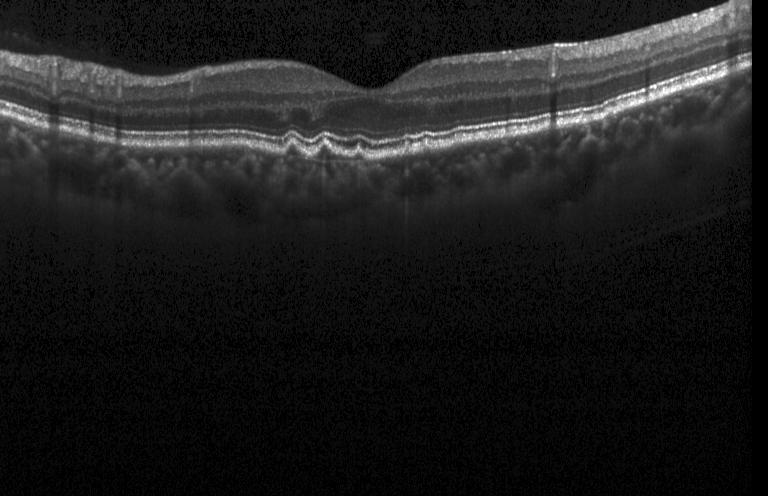

Optical coherence tomography scan, spectral-domain optical coherence tomography, instrument: Heidelberg Spectralis, macular scan
Diagnosis: drusen.